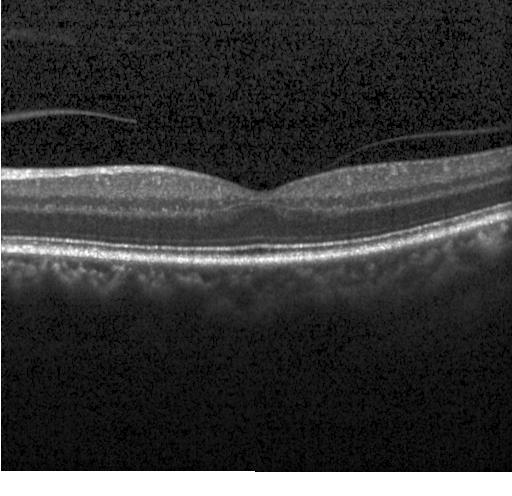

Retinal OCT B-scan · instrument: Heidelberg Spectralis · through the macula
Finding: neither CNV, DME, nor drusen.